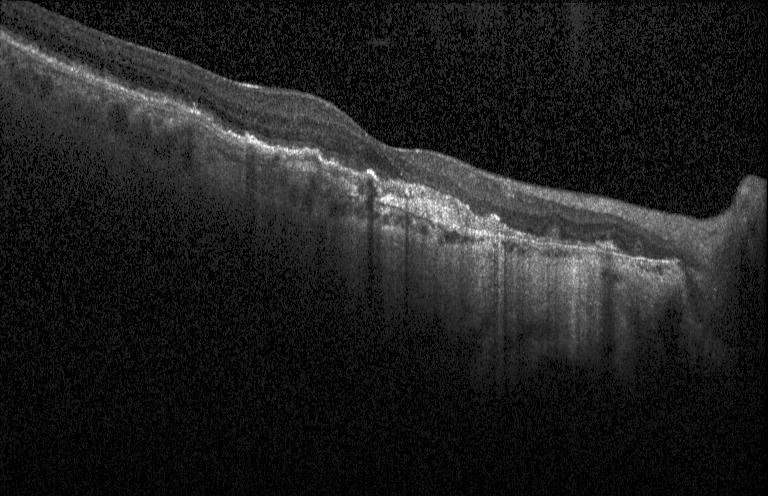 Retinal OCT cross-section showing a choroidal neovascular membrane.